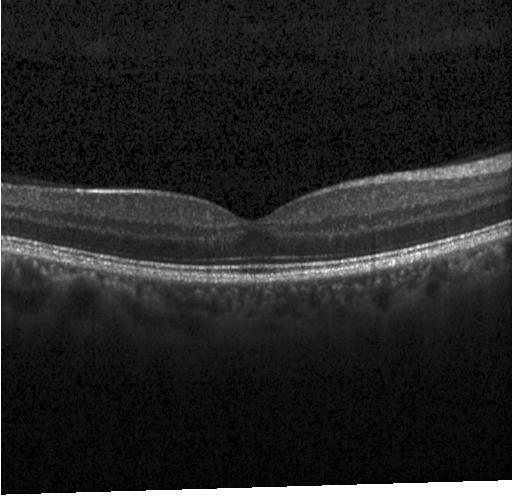

Optical coherence tomography B-scan · SD-OCT · Heidelberg Spectralis · macular scan — Macular OCT: no choroidal neovascularization, diabetic macular edema, or drusen.